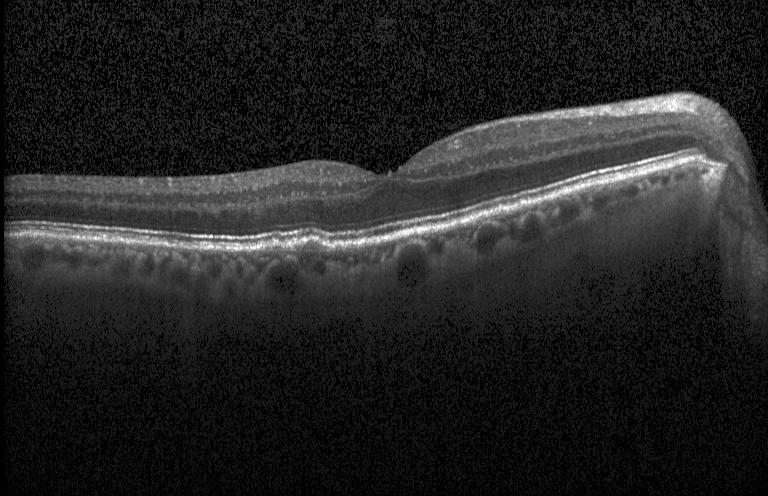 OCT line scan · fovea-centered. The scan shows sub-RPE drusenoid deposits.